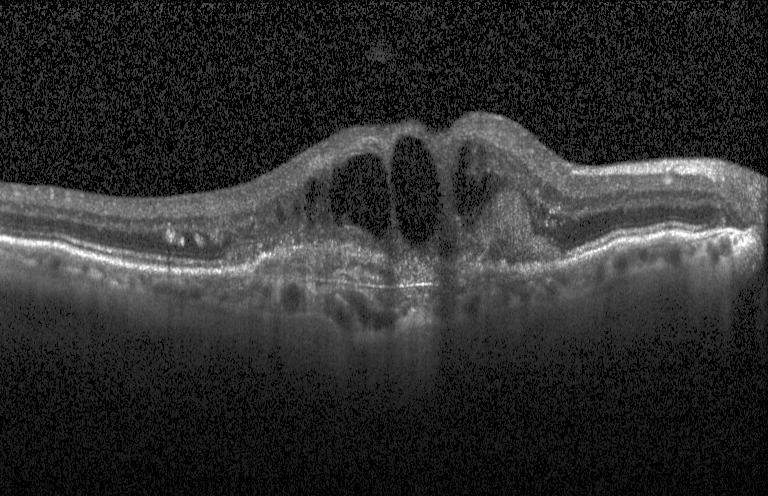 Retinal OCT B-scan.
Finding: a choroidal neovascular membrane.